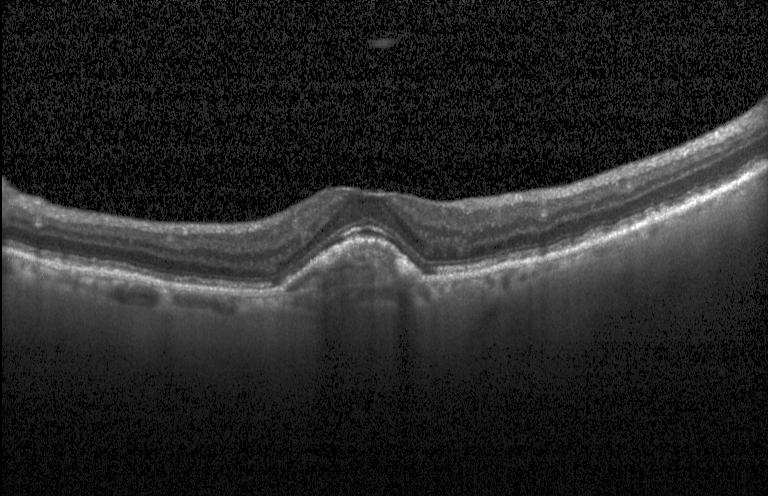

Optical coherence tomography B-scan; instrument: Heidelberg Spectralis; fovea-centered — The scan shows choroidal neovascularization.